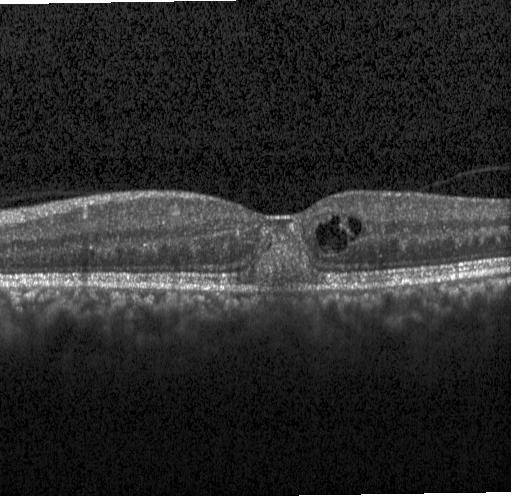
Through the macula, retinal OCT cross-section, SD-OCT — The scan shows choroidal neovascularization (CNV).